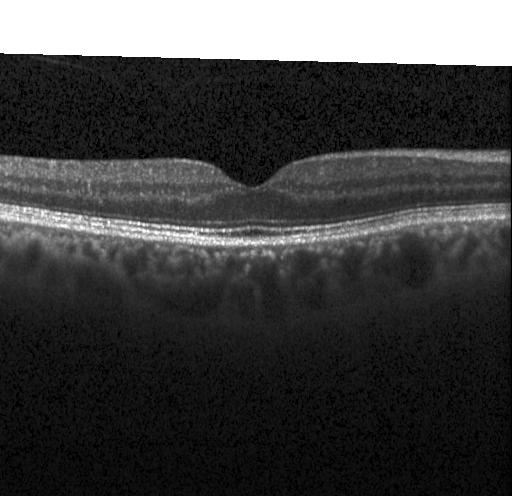

Instrument: Heidelberg Spectralis. Retinal OCT B-scan — Finding: no evidence of choroidal neovascularization, diabetic macular edema, or drusen.